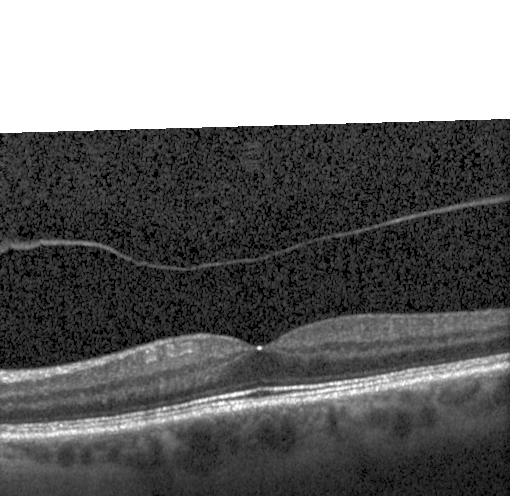
Diagnosis: no evidence of choroidal neovascularization, diabetic macular edema, or drusen.